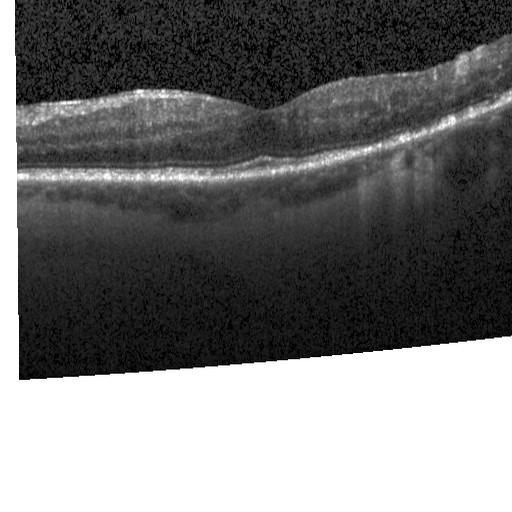 Spectral-domain OCT B-scan: diabetic macular edema.